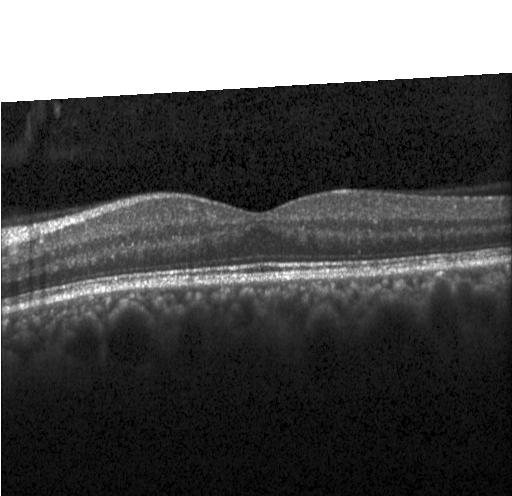

Retinal OCT cross-section. This B-scan demonstrates no CNV, no DME, and no drusen.